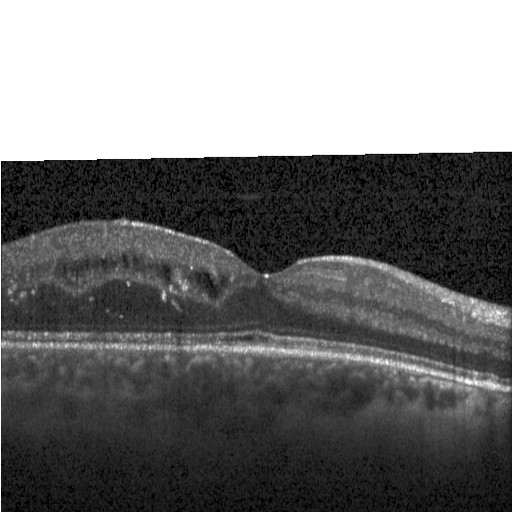

Macular OCT demonstrating diabetic macular edema (DME).